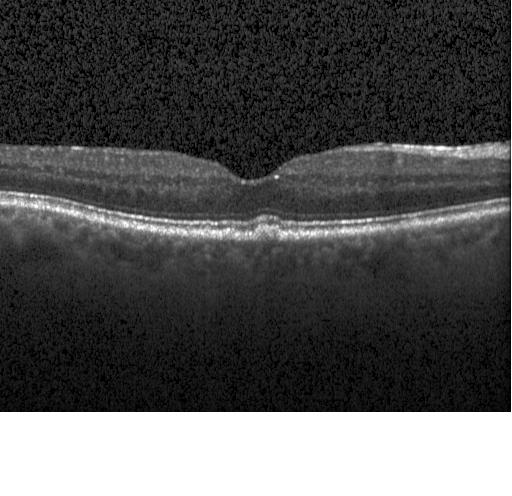

OCT scan showing drusen.